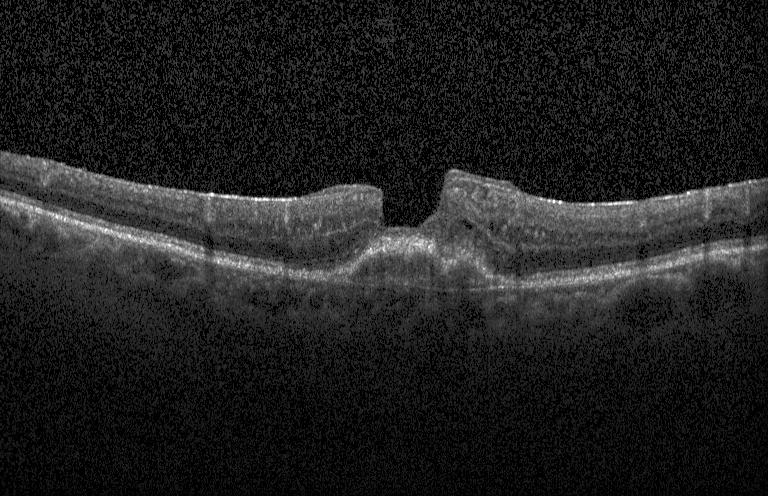
Spectral-domain OCT; OCT B-scan; instrument: Heidelberg Spectralis; through the macula. Finding: choroidal neovascularization (CNV).